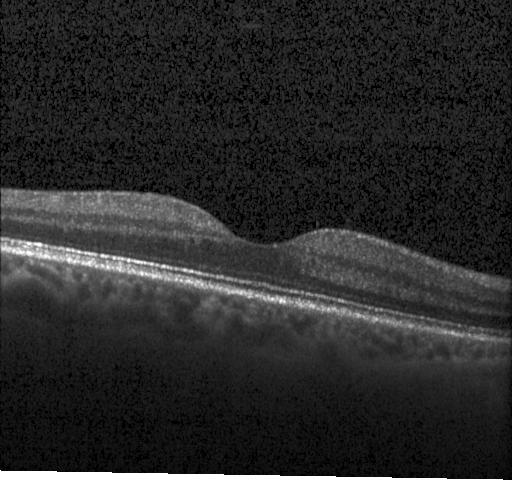
Finding: no evidence of CNV, DME, or drusen.